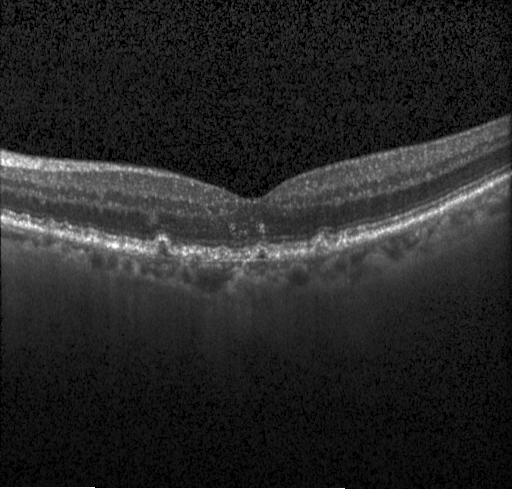
Diagnosis: a choroidal neovascular membrane.